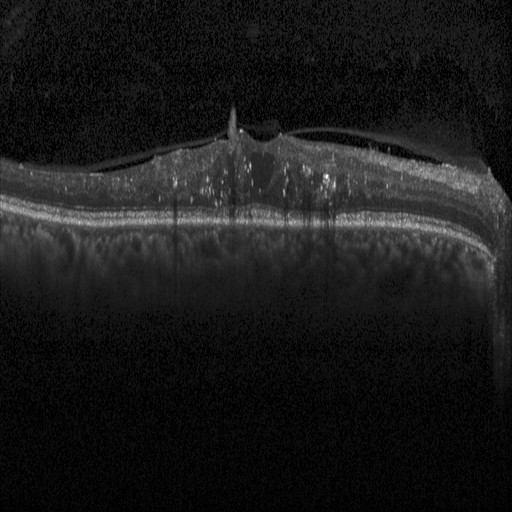
Impression: diabetic macular edema.